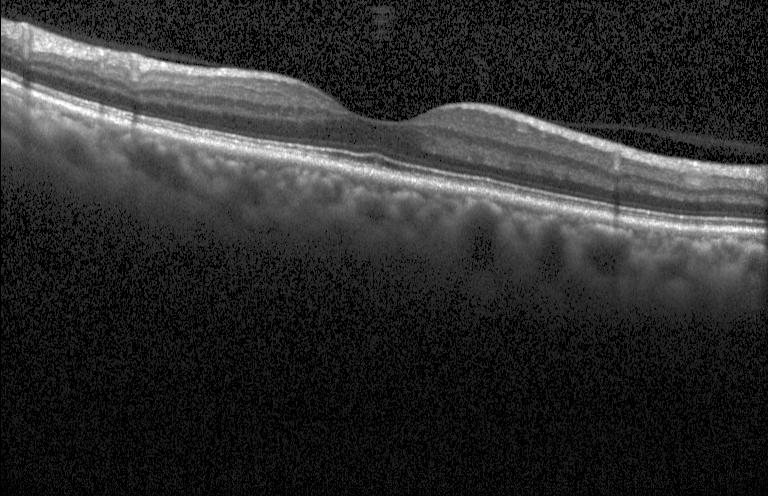
Optical coherence tomography B-scan · spectral-domain OCT. OCT finding: no CNV, no DME, and no drusen.